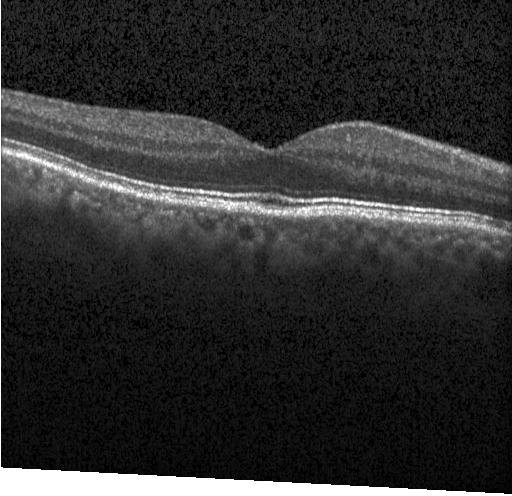
SD-OCT. Optical coherence tomography scan. Horizontal scan through the fovea. Assessment: no choroidal neovascularization, diabetic macular edema, or drusen.